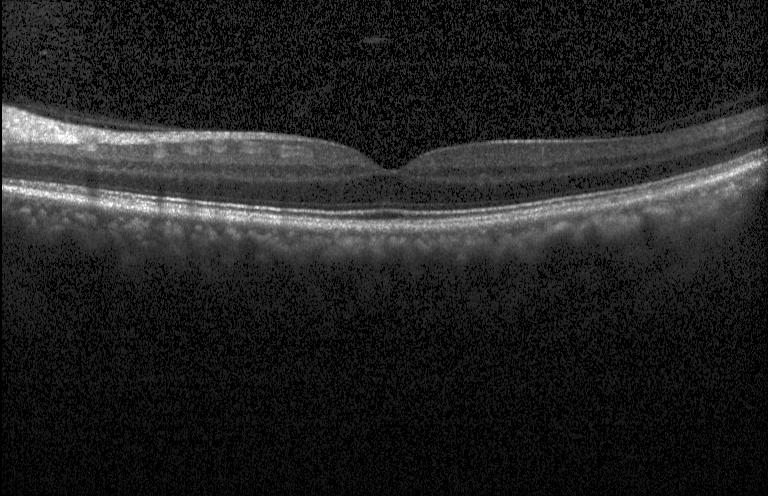

SD-OCT; OCT B-scan; instrument: Heidelberg Spectralis
Impression: no evidence of choroidal neovascularization, diabetic macular edema, or drusen.